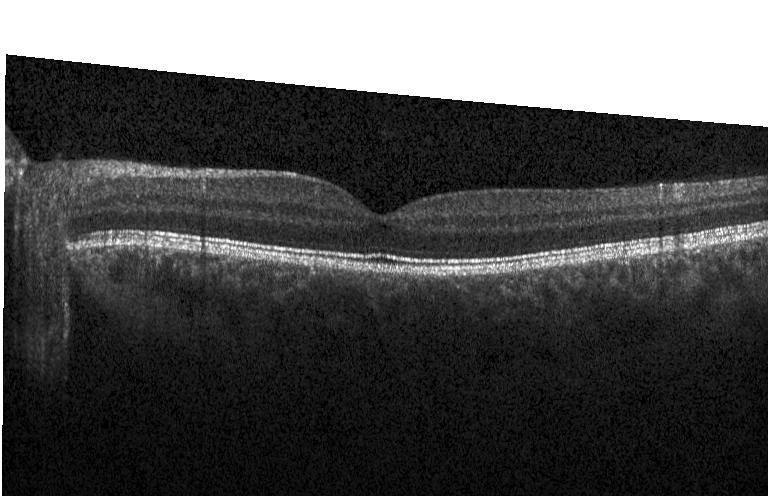 Assessment: neither choroidal neovascularization, diabetic macular edema, nor drusen.